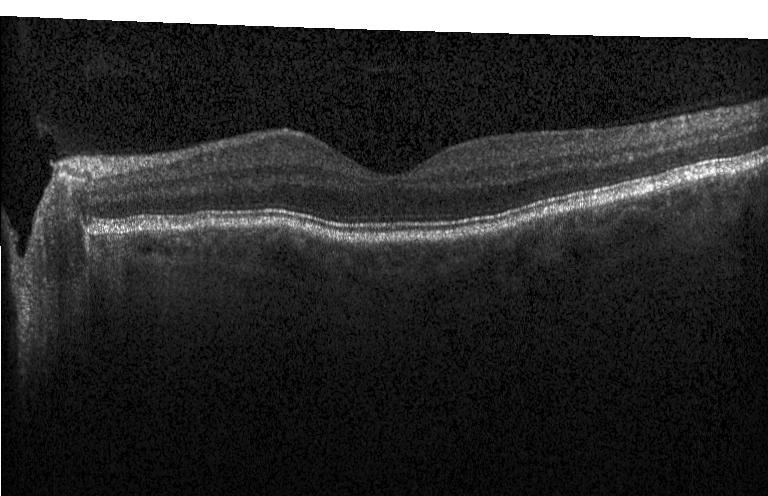
Optical coherence tomography scan · Heidelberg Spectralis OCT system. Diagnosis: no choroidal neovascularization, no diabetic macular edema, and no drusen.